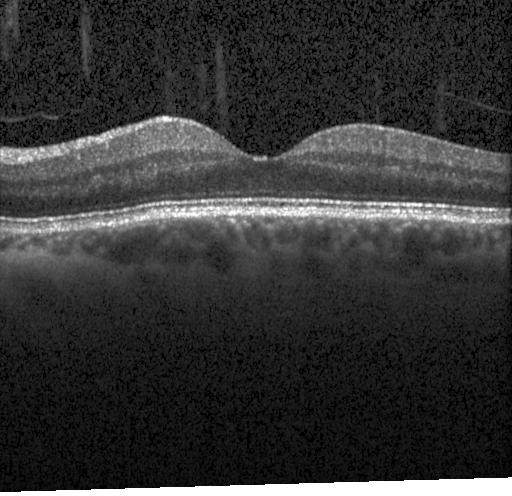 Instrument: Heidelberg Spectralis; SD-OCT; through the macula; OCT B-scan
Dx: no choroidal neovascularization, no diabetic macular edema, and no drusen.